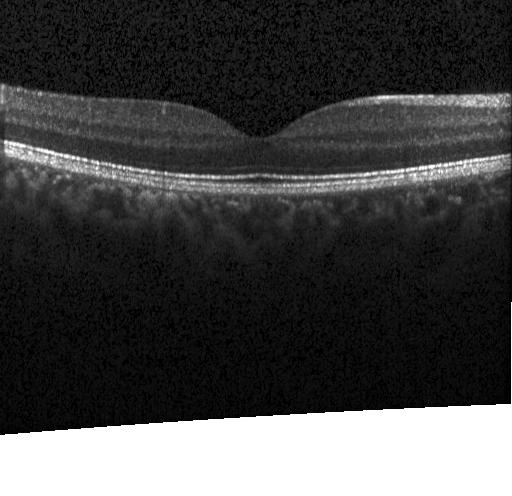
Centered on the fovea; retinal OCT cross-section. OCT finding: no choroidal neovascularization, diabetic macular edema, or drusen.